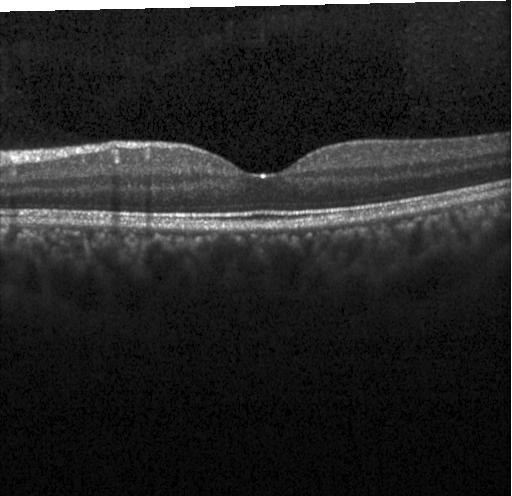 No evidence of choroidal neovascularization, diabetic macular edema, or drusen.